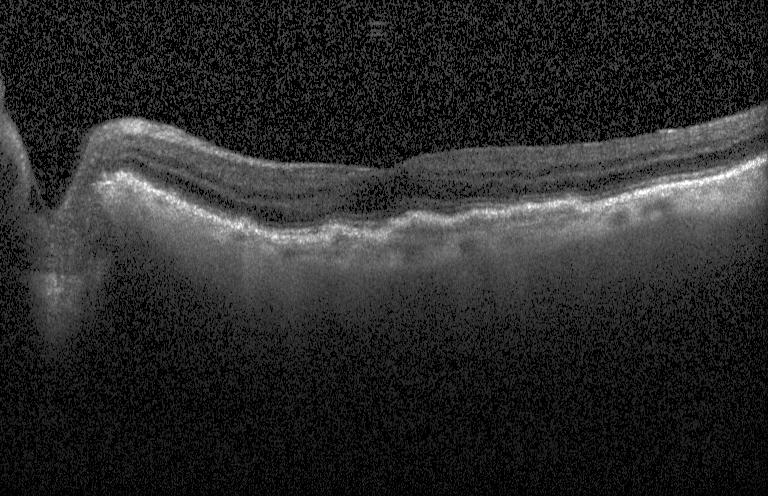

Diagnosis: a choroidal neovascular membrane.